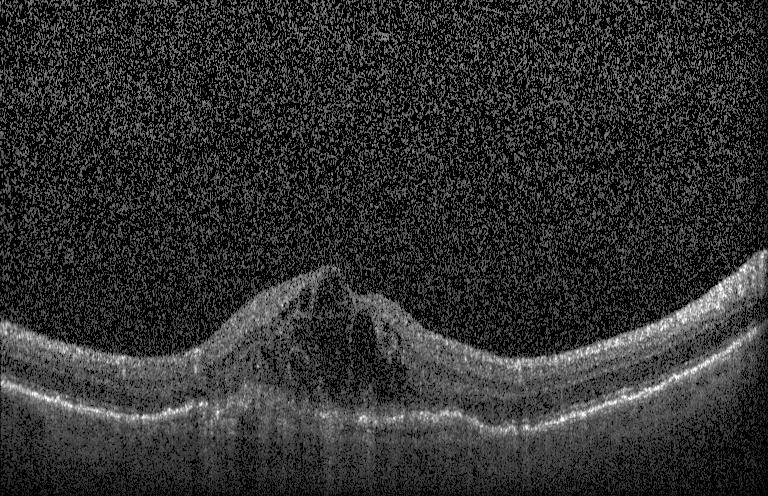

Acquired on a Heidelberg Spectralis; SD-OCT; retinal OCT cross-section — Assessment: choroidal neovascularization.